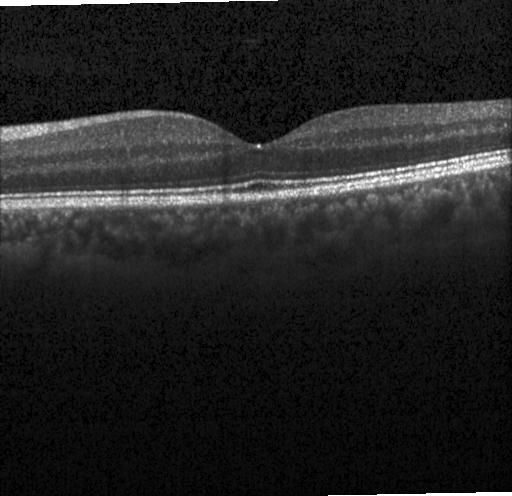 Heidelberg Spectralis; horizontal scan through the fovea; retinal OCT cross-section — No evidence of CNV, DME, or drusen.